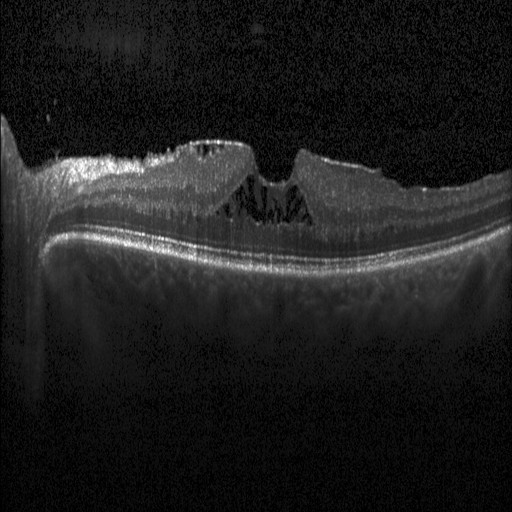
Through the macula. Retinal OCT B-scan.
Finding: DME.